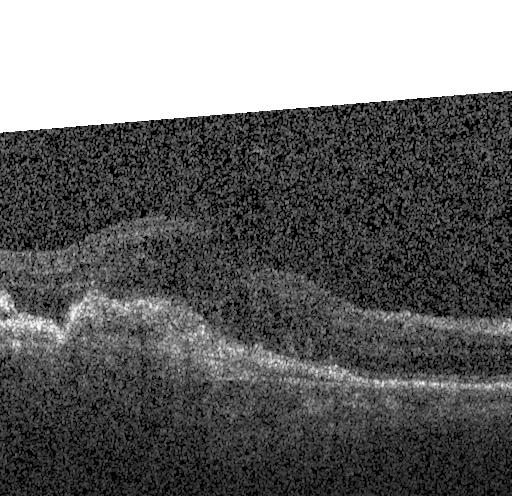 Optical coherence tomography B-scan
Finding: CNV.